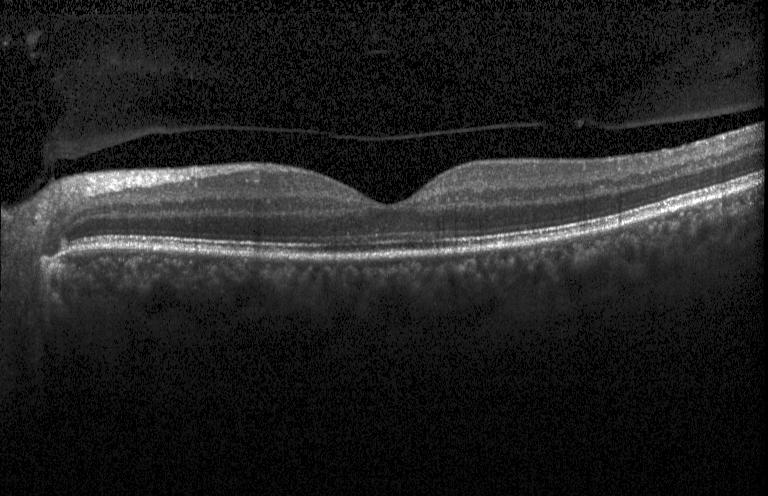
Retinal OCT B-scan.
Assessment: no CNV, no DME, and no drusen.